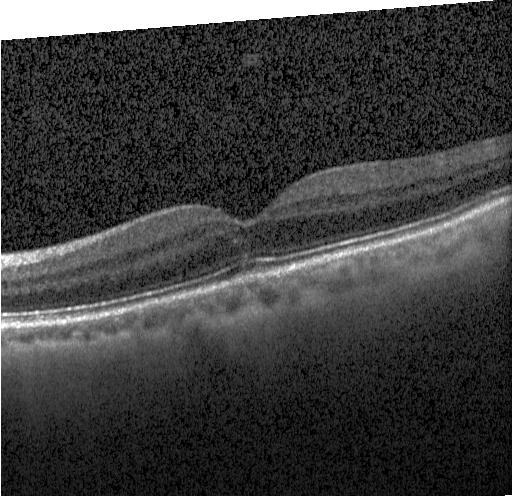
Macular OCT demonstrating no choroidal neovascularization, diabetic macular edema, or drusen.